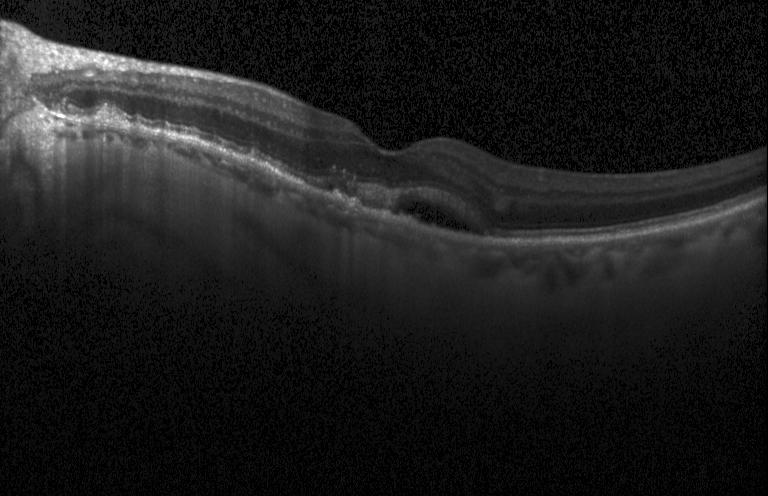 Centered on the fovea · SD-OCT · acquired on a Heidelberg Spectralis · OCT line scan
Impression: a choroidal neovascular membrane.